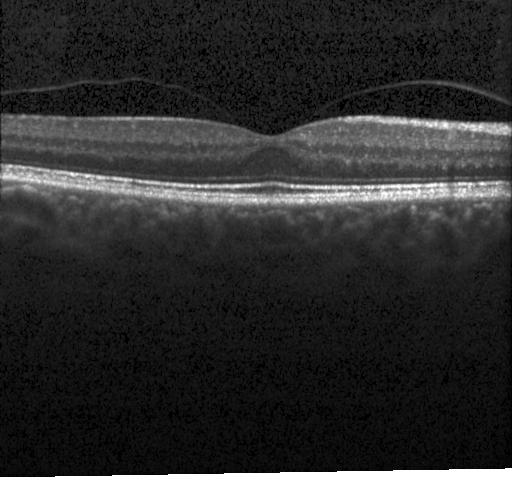

Impression: no choroidal neovascularization, no diabetic macular edema, and no drusen.